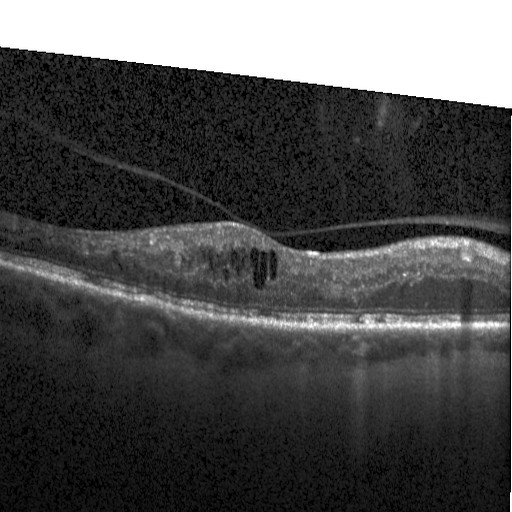

OCT scan showing diabetic macular edema (DME).